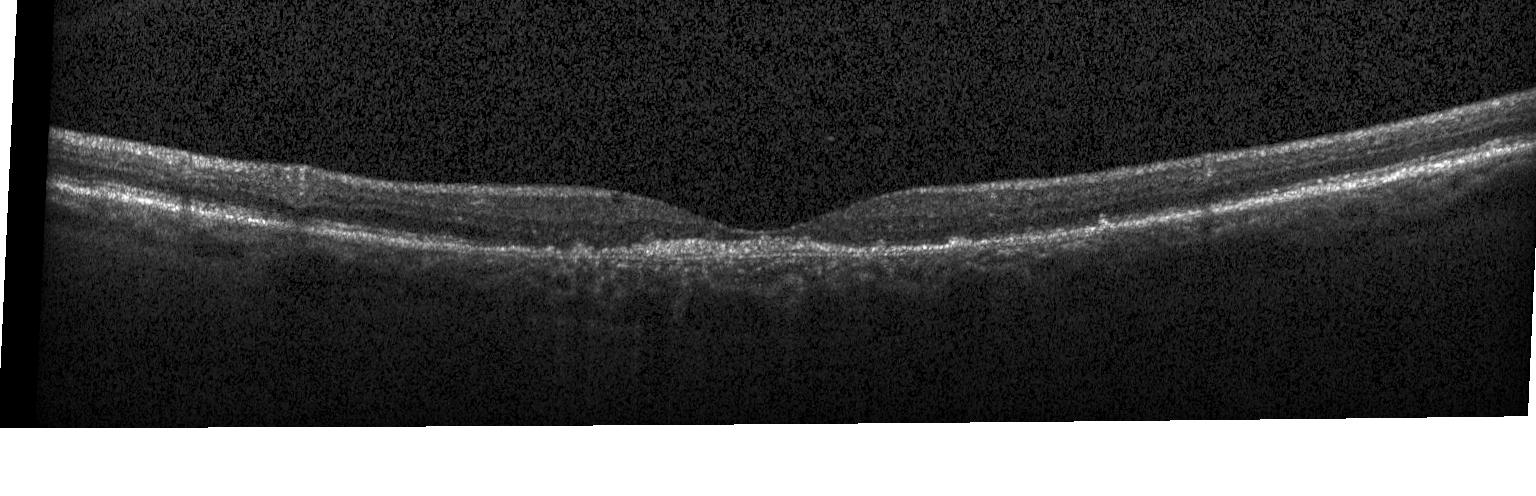
OCT scan showing CNV.